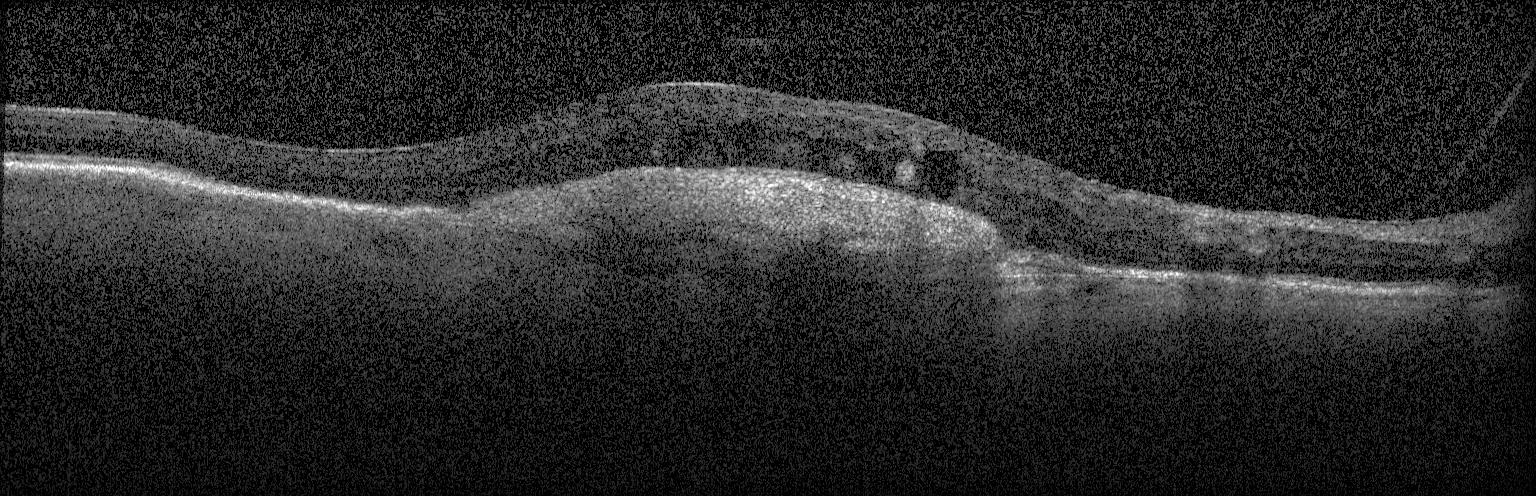

Retinal OCT cross-section. This B-scan demonstrates a choroidal neovascular membrane.